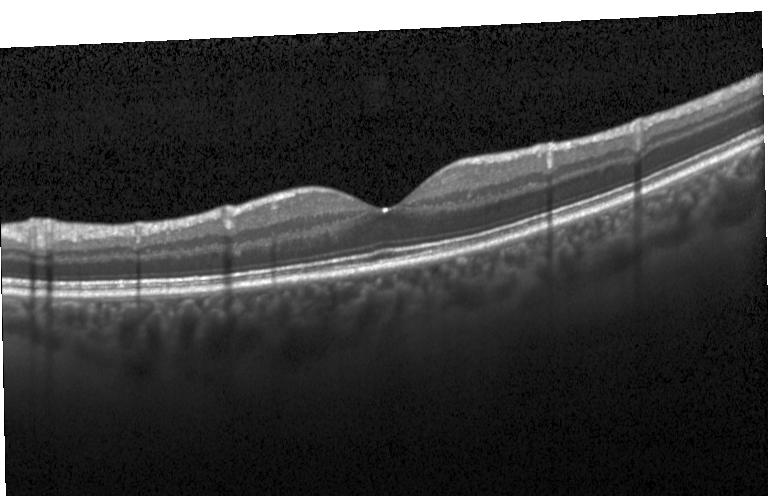

Retinal OCT cross-section showing neither choroidal neovascularization, diabetic macular edema, nor drusen.